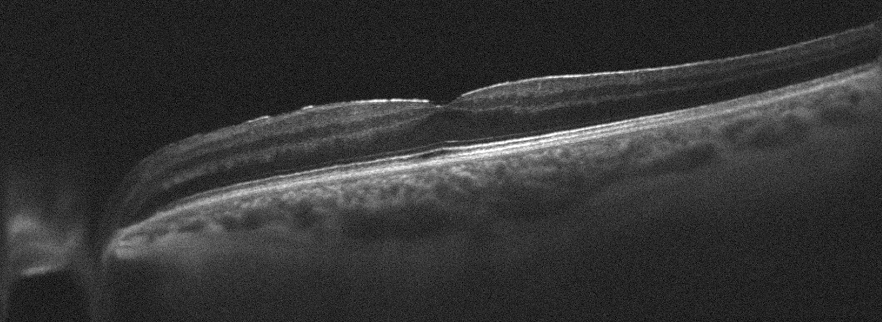

Instrument: Optovue Avanti RTVue XR, oculus sinister, OCT B-scan, macular scan — Impression: epiretinal membrane (ERM).